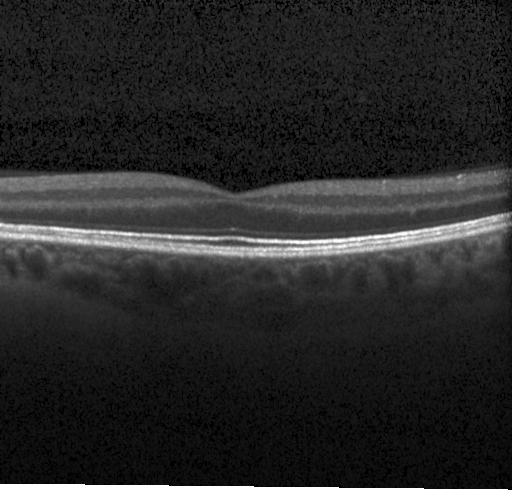 Retinal OCT B-scan; Heidelberg Spectralis — Assessment: neither choroidal neovascularization, diabetic macular edema, nor drusen.